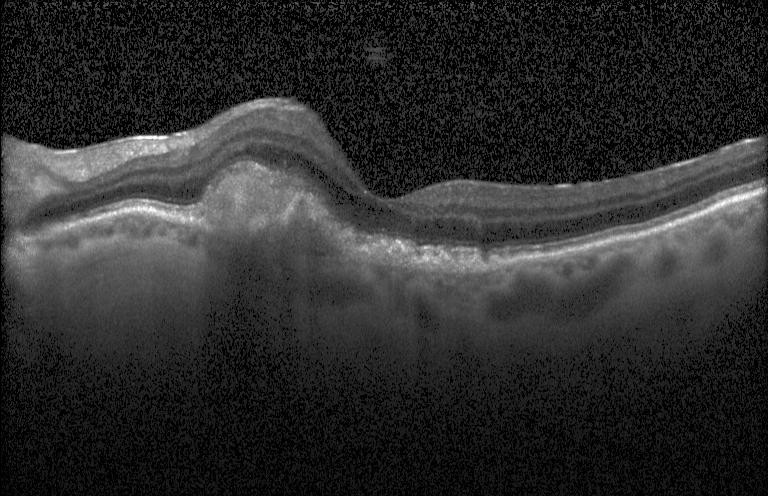

Optical coherence tomography B-scan.
Finding: choroidal neovascularization (CNV).